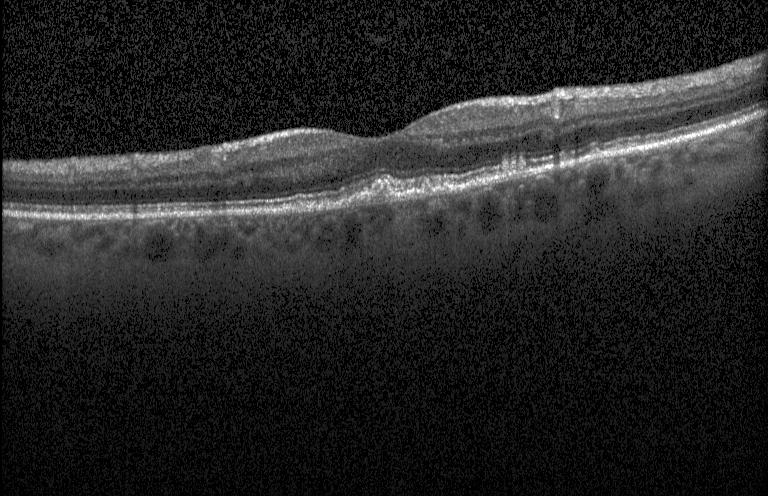 Finding: multiple drusen.